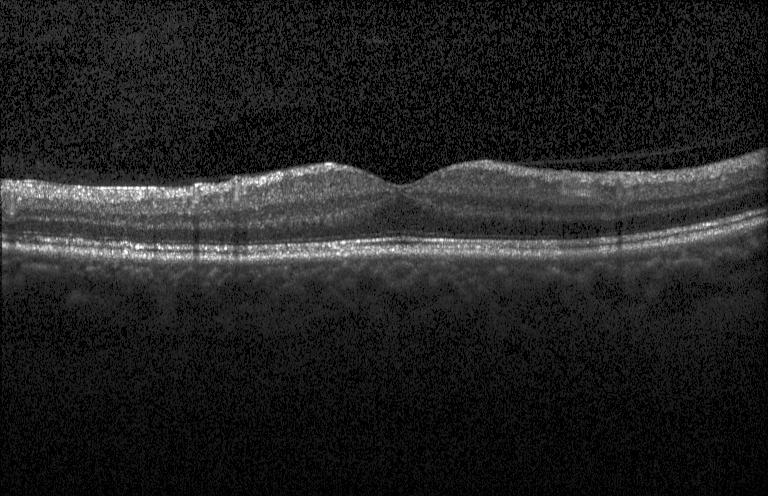 This B-scan demonstrates no CNV, no DME, and no drusen.